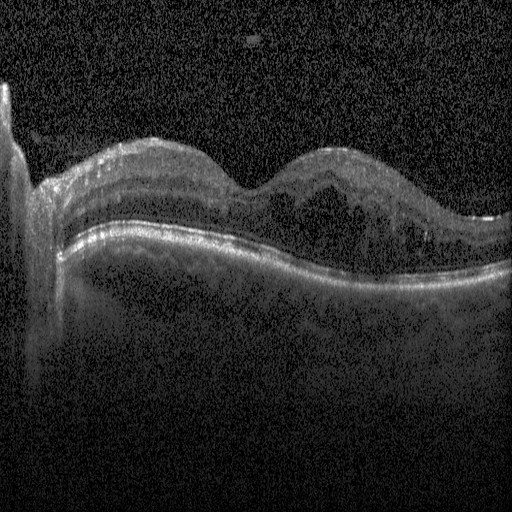

Finding: diabetic macular edema.